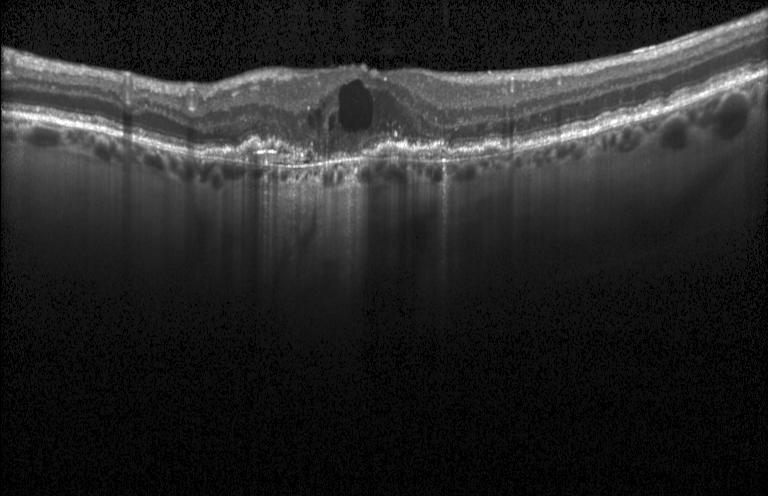

OCT line scan · macular scan · acquired on a Heidelberg Spectralis · spectral-domain OCT
This B-scan demonstrates CNV.